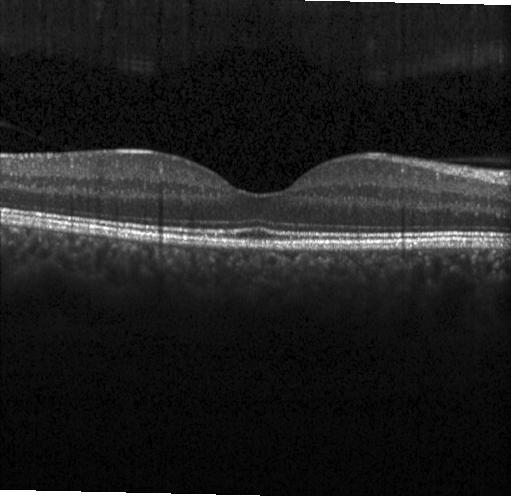

OCT scan showing no choroidal neovascularization, diabetic macular edema, or drusen.